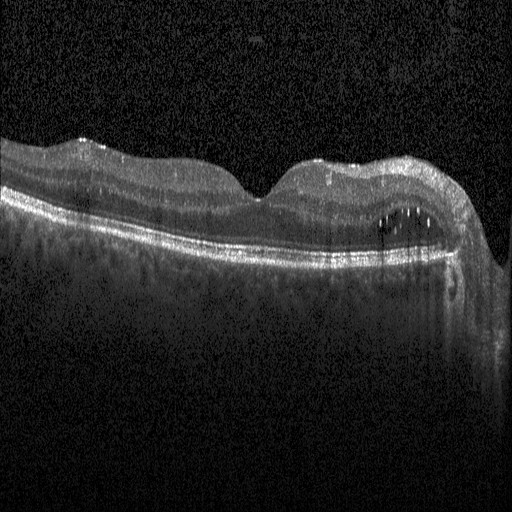 Spectral-domain optical coherence tomography, fovea-centered, retinal OCT cross-section, Heidelberg Spectralis — The scan shows diabetic macular edema (DME).